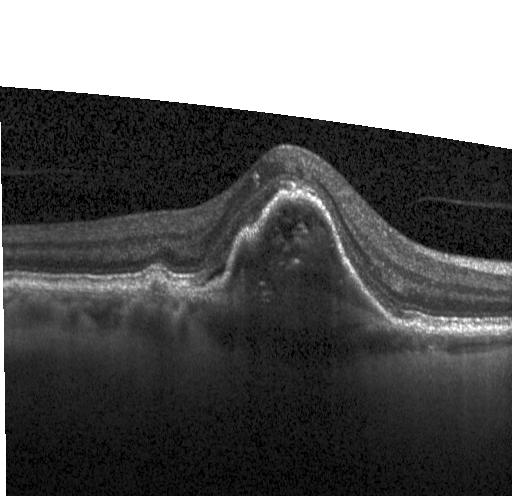
Heidelberg Spectralis. Spectral-domain optical coherence tomography. Horizontal scan through the fovea. Retinal OCT cross-section — Impression: a choroidal neovascular membrane.